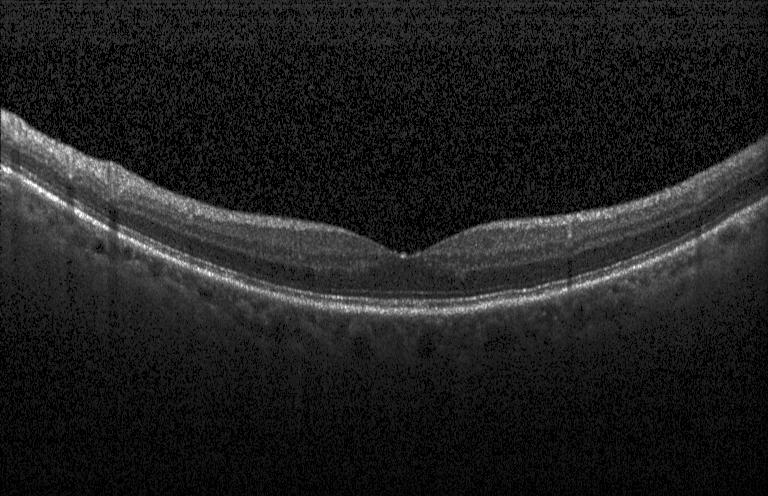 Retinal OCT cross-section. Spectral-domain OCT. Through the macula.
No CNV, DME, or drusen.